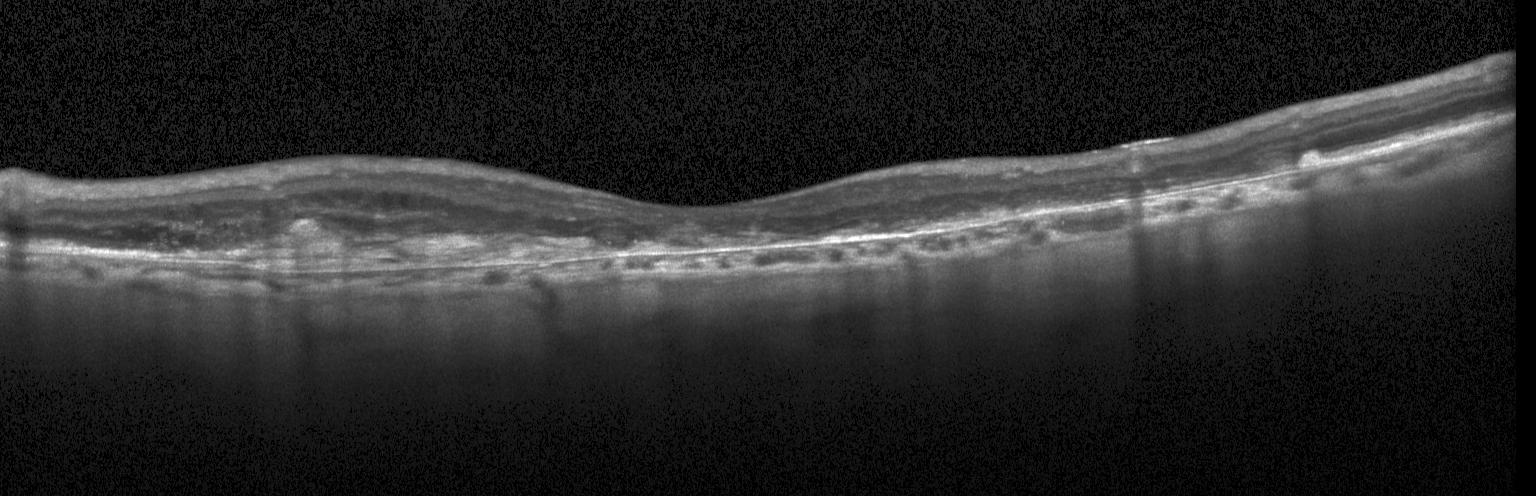
OCT line scan; spectral-domain OCT
Macular OCT: choroidal neovascularization.